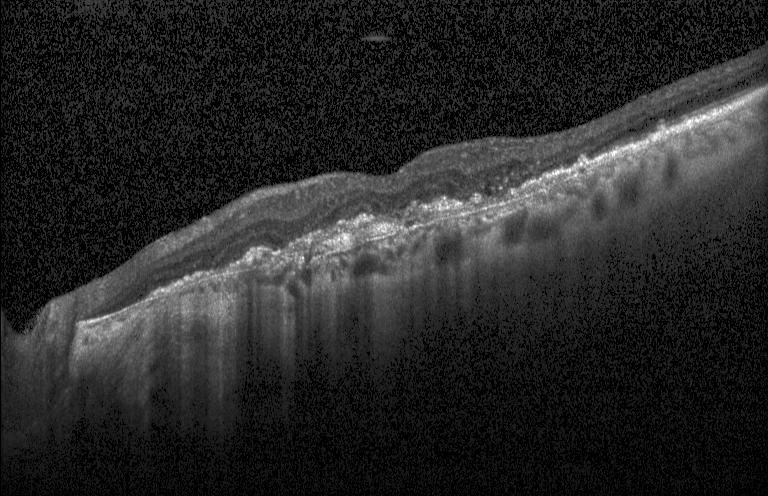 Spectral-domain OCT. OCT line scan.
Dx: a choroidal neovascular membrane.